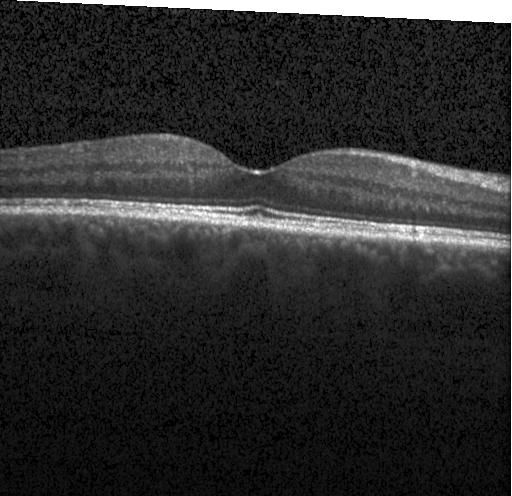 Macular OCT demonstrating no evidence of CNV, DME, or drusen.